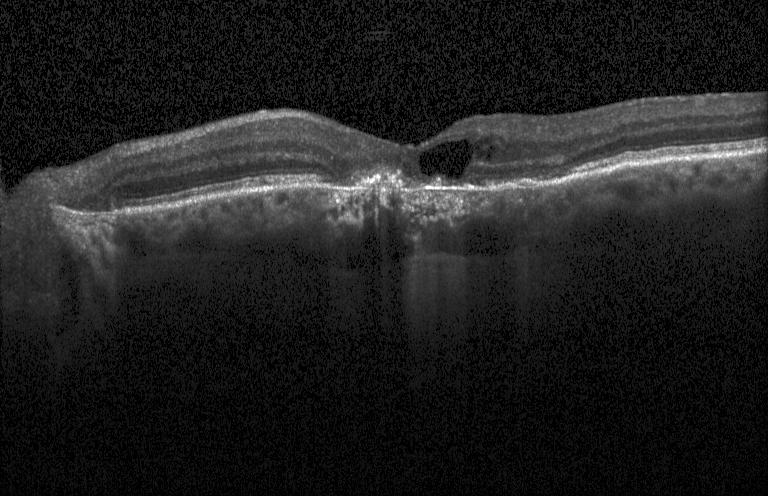

Diagnosis: a choroidal neovascular membrane.